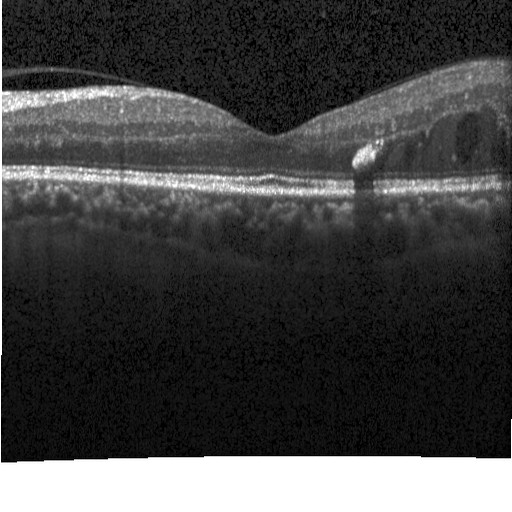 Through the macula; instrument: Heidelberg Spectralis; optical coherence tomography scan. Diabetic macular edema (DME).